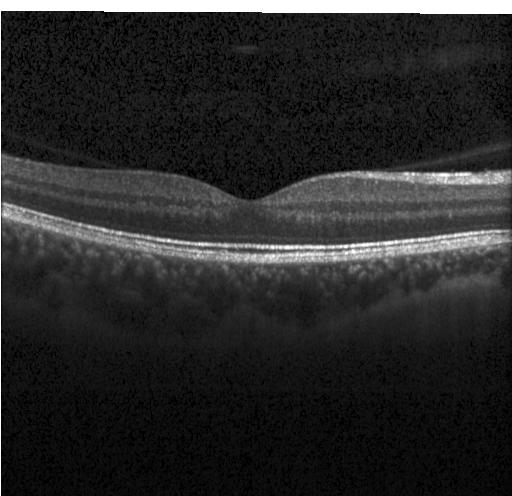 Macular scan. Spectral-domain OCT. OCT line scan — Finding: no CNV, DME, or drusen.